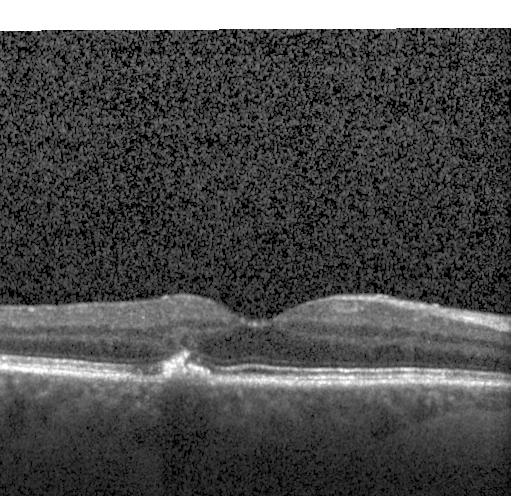

Heidelberg Spectralis, optical coherence tomography scan, horizontal scan through the fovea.
Finding: multiple drusen.